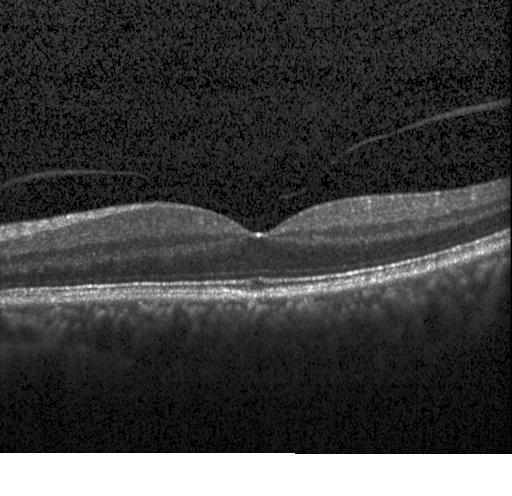
Assessment: no evidence of choroidal neovascularization, diabetic macular edema, or drusen.